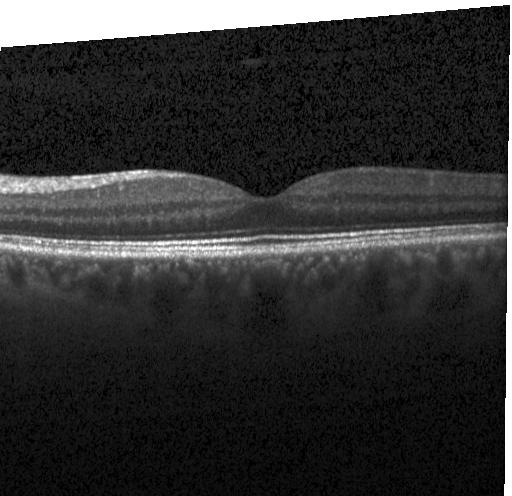

Spectral-domain OCT · horizontal scan through the fovea · acquired on a Heidelberg Spectralis · optical coherence tomography scan — OCT finding: neither CNV, DME, nor drusen.